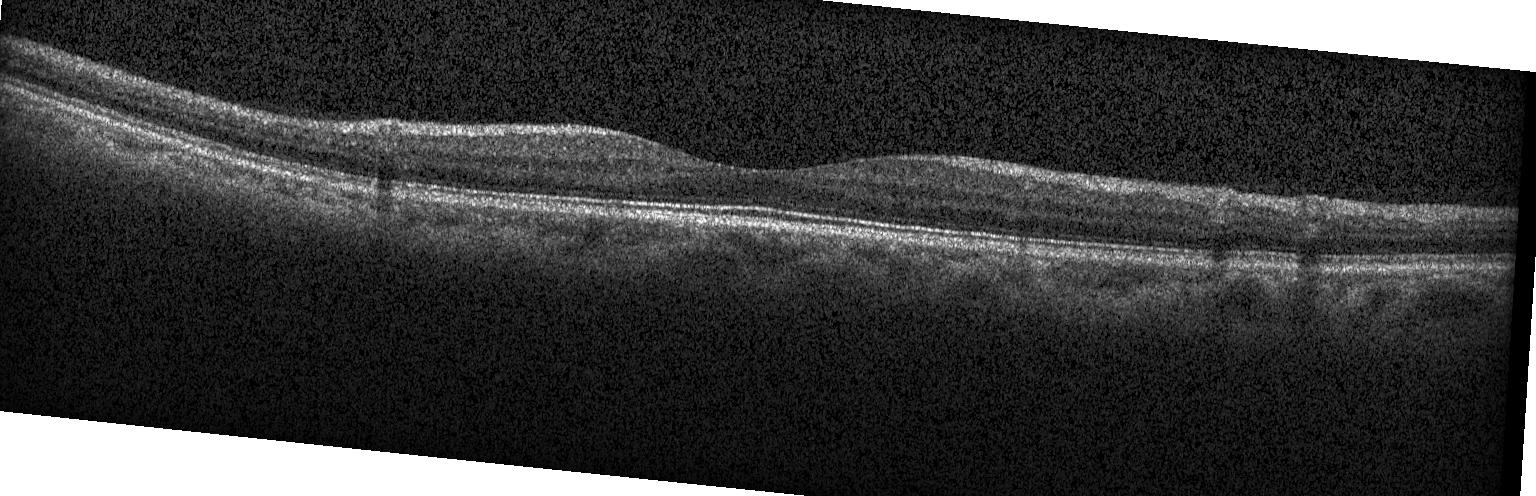

Diagnosis: no evidence of CNV, DME, or drusen.